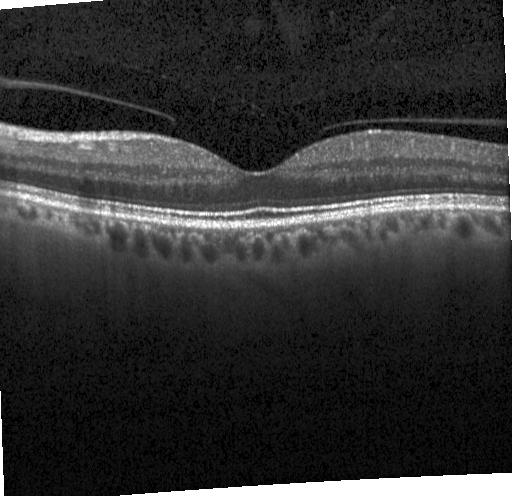
Spectral-domain OCT B-scan: no choroidal neovascularization, diabetic macular edema, or drusen.